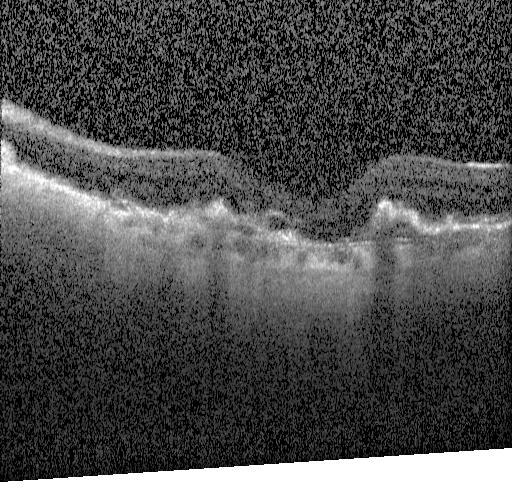

OCT B-scan showing a choroidal neovascular membrane.